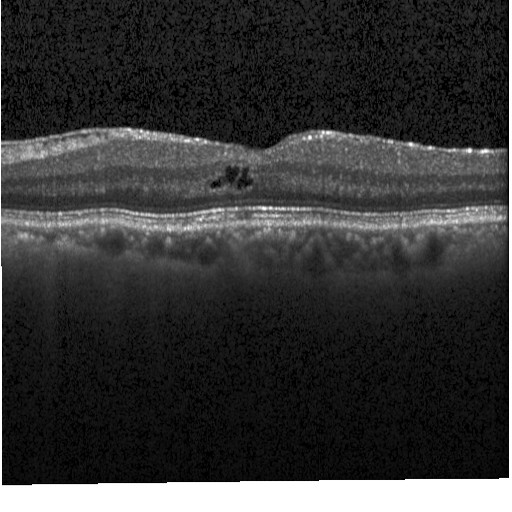 SD-OCT; through the macula; retinal OCT cross-section.
This B-scan demonstrates diabetic macular edema.